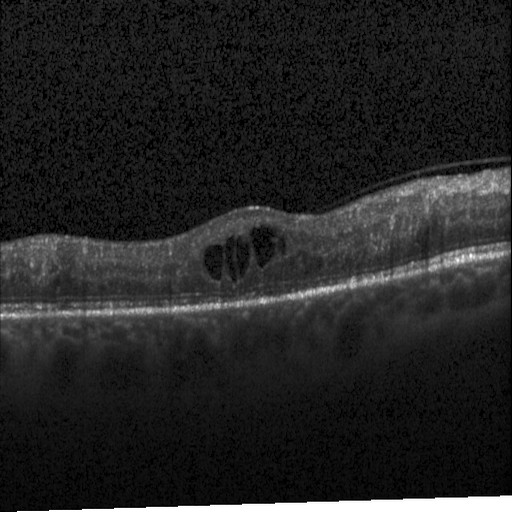 Impression: diabetic macular edema.